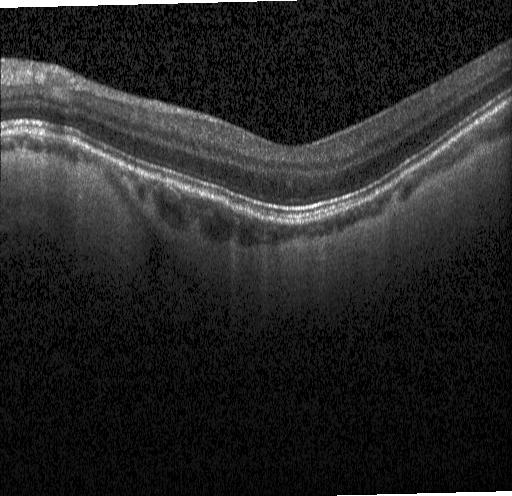

Optical coherence tomography scan. Finding: no CNV, DME, or drusen.